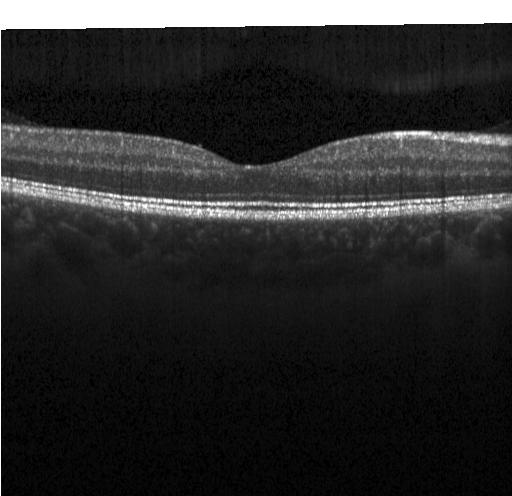 Retinal OCT cross-section.
Macular OCT: neither choroidal neovascularization, diabetic macular edema, nor drusen.